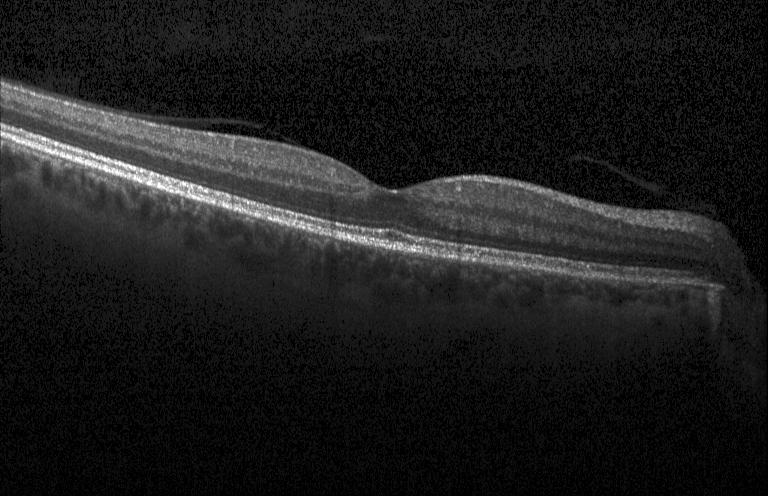

Macular OCT: neither choroidal neovascularization, diabetic macular edema, nor drusen.